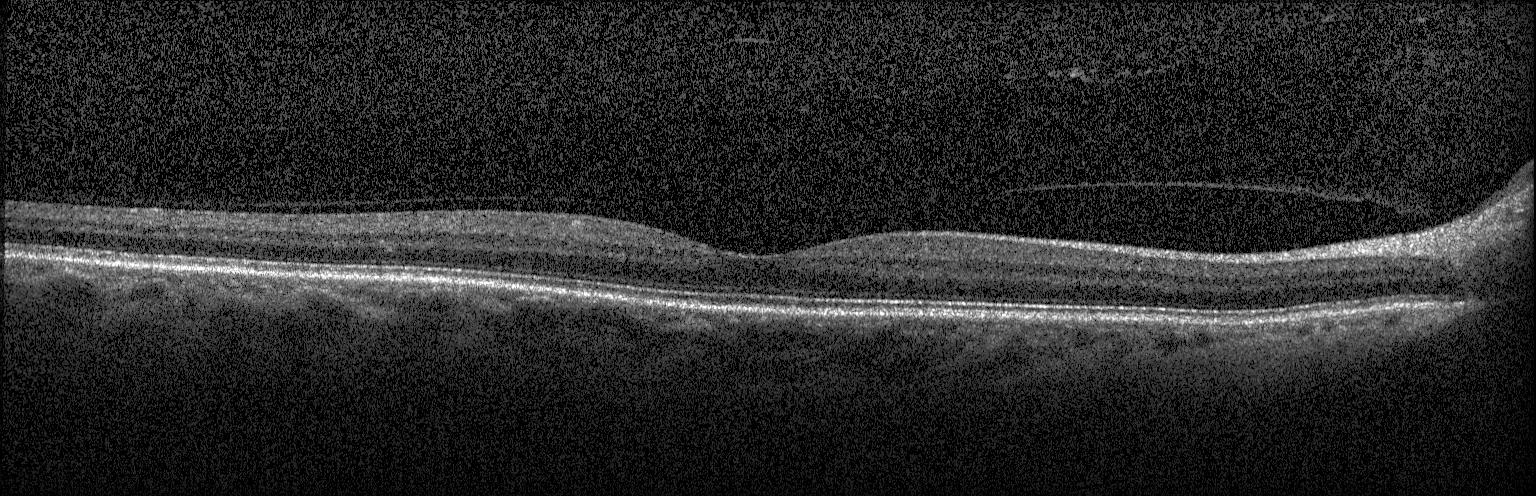 OCT B-scan, spectral-domain optical coherence tomography, Heidelberg Spectralis OCT system — This B-scan demonstrates neither choroidal neovascularization, diabetic macular edema, nor drusen.